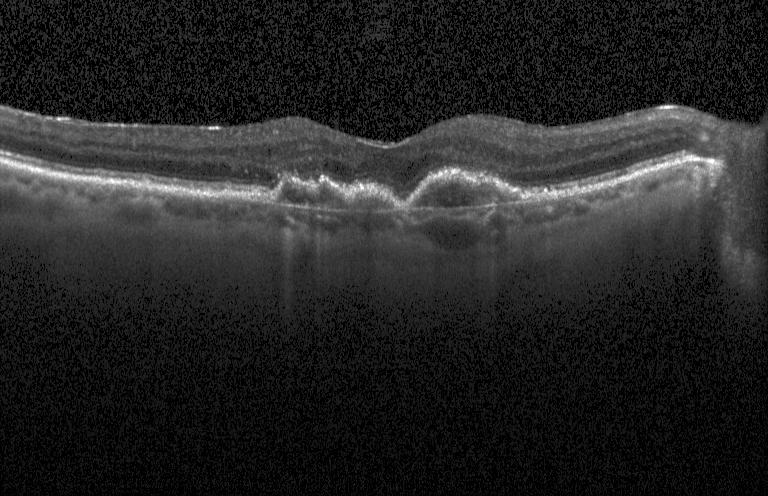
Heidelberg Spectralis. Horizontal scan through the fovea. OCT line scan
Choroidal neovascularization.